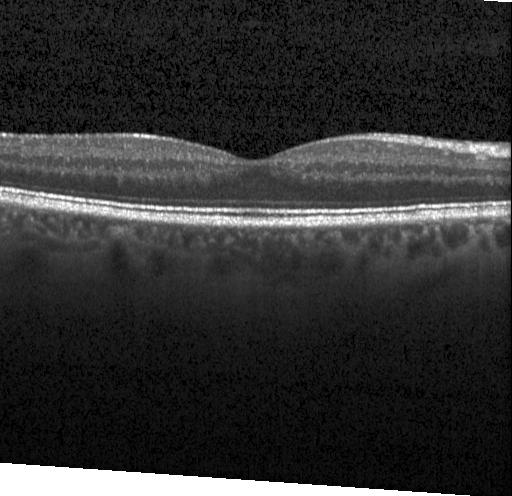
Macular OCT: no evidence of choroidal neovascularization, diabetic macular edema, or drusen.